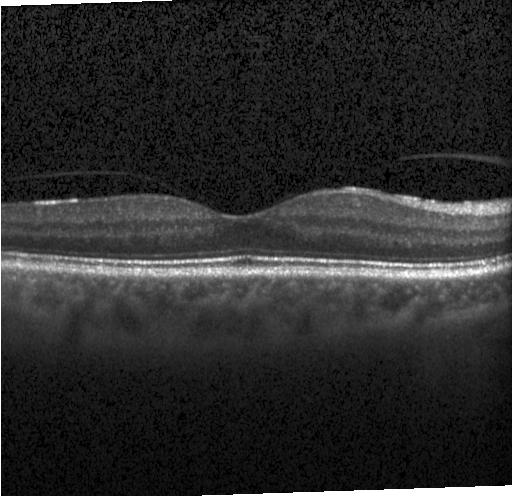
The scan shows neither choroidal neovascularization, diabetic macular edema, nor drusen.